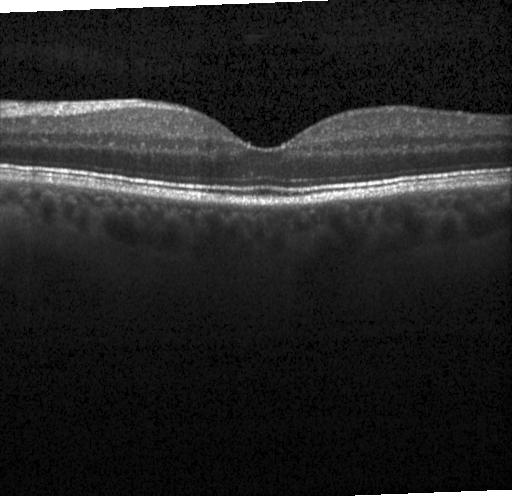 Retinal OCT B-scan.
Macular OCT: no choroidal neovascularization, no diabetic macular edema, and no drusen.